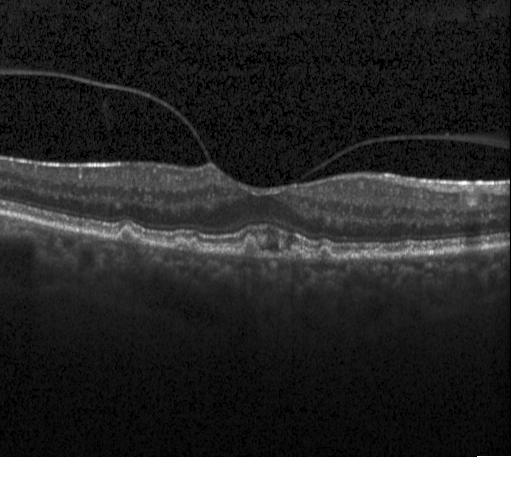 Retinal OCT cross-section showing drusen.